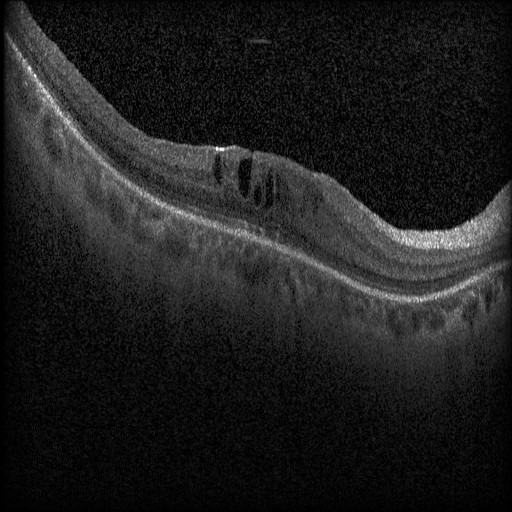

OCT line scan · Heidelberg Spectralis OCT system.
Diabetic macular edema.